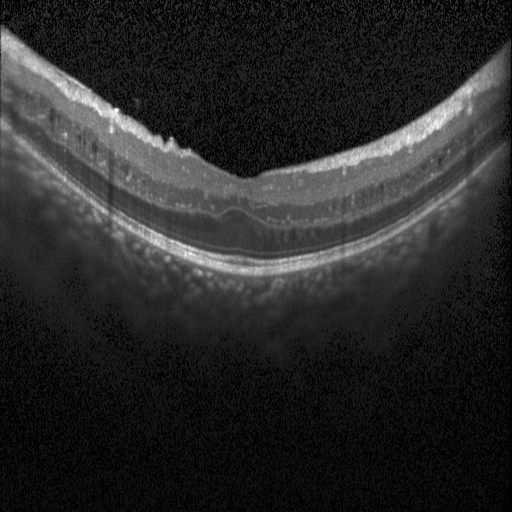
SD-OCT, OCT B-scan. Diagnosis: diabetic macular edema (DME).